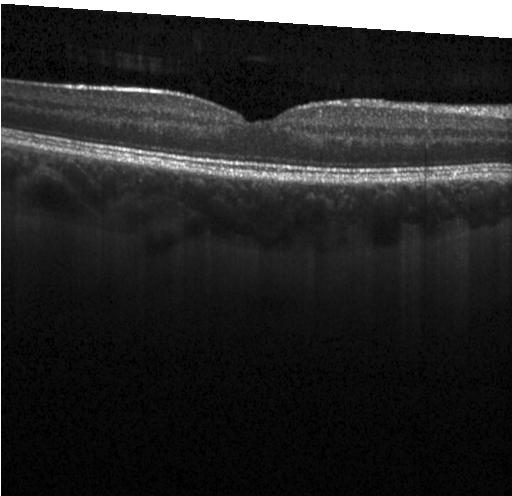
Retinal OCT cross-section · through the macula · SD-OCT · instrument: Heidelberg Spectralis
The scan shows neither choroidal neovascularization, diabetic macular edema, nor drusen.